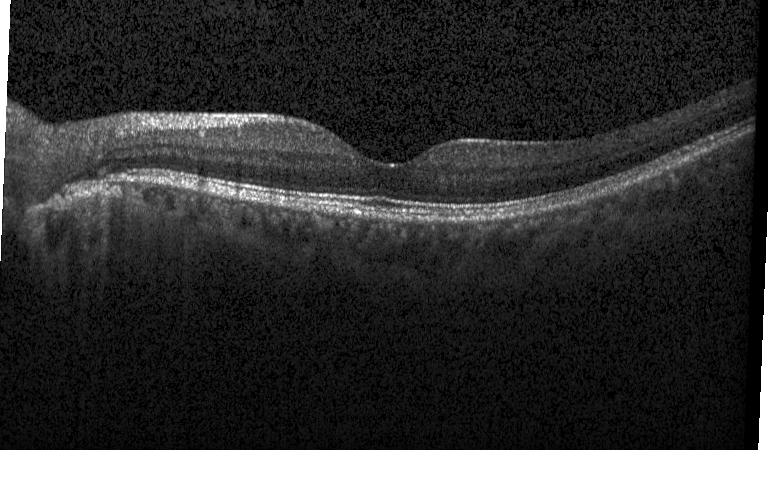

OCT B-scan showing neither choroidal neovascularization, diabetic macular edema, nor drusen.